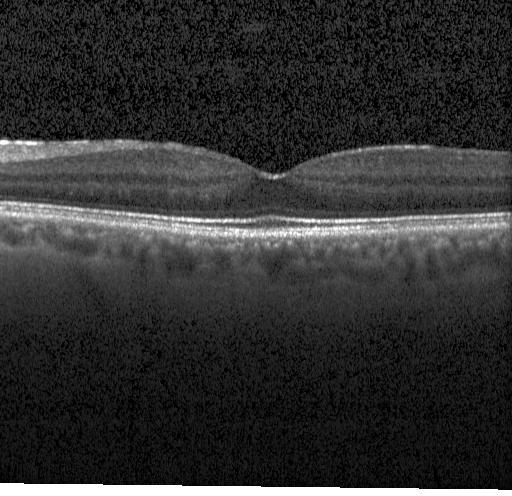

OCT scan showing no evidence of CNV, DME, or drusen.